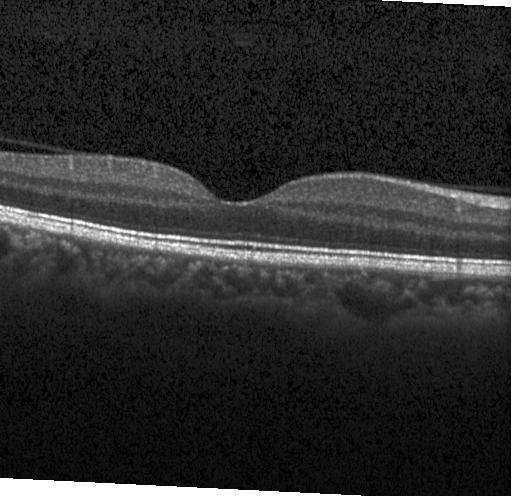
This B-scan demonstrates neither choroidal neovascularization, diabetic macular edema, nor drusen.